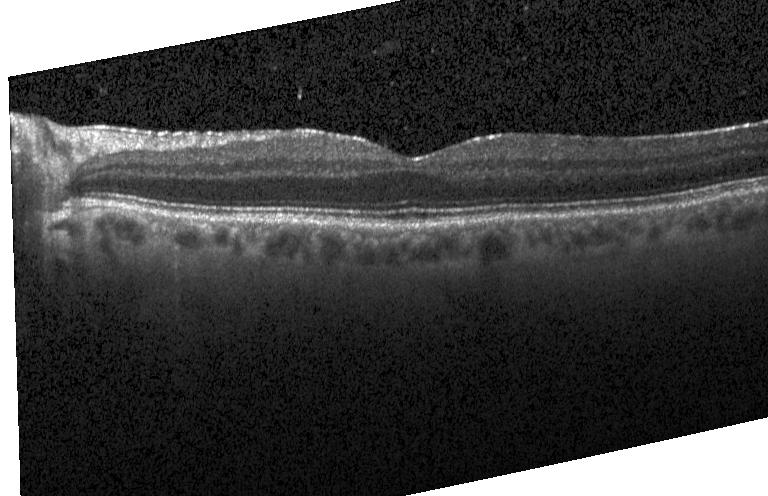

Finding: no CNV, no DME, and no drusen.